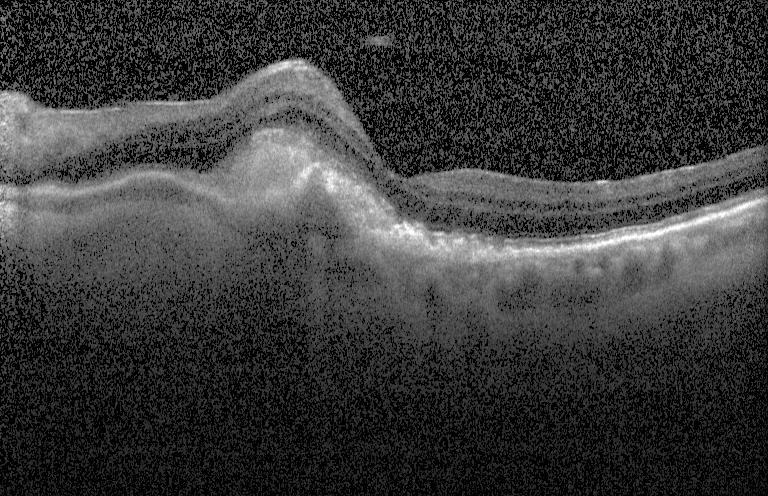
Acquired on a Heidelberg Spectralis · through the macula · OCT line scan
Macular OCT: a choroidal neovascular membrane.